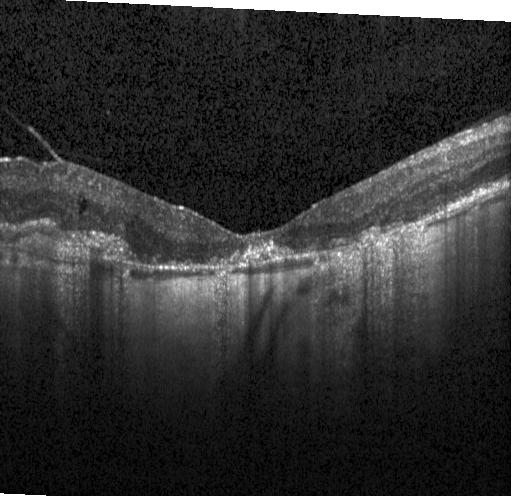

OCT B-scan showing choroidal neovascularization.